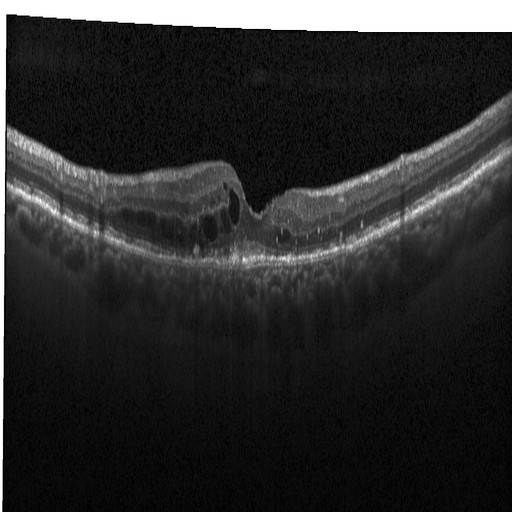
OCT line scan · acquired on a Heidelberg Spectralis — Impression: DME.